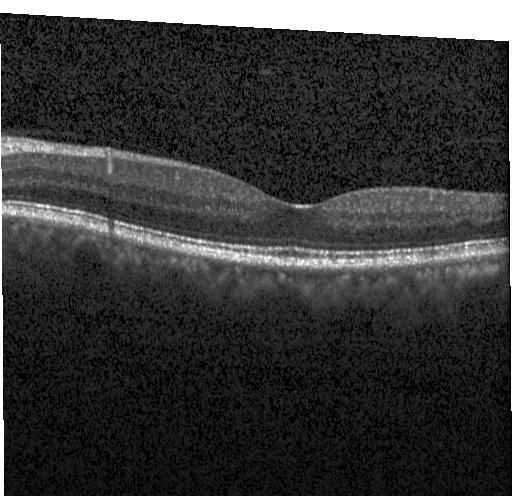 Dx: neither choroidal neovascularization, diabetic macular edema, nor drusen.